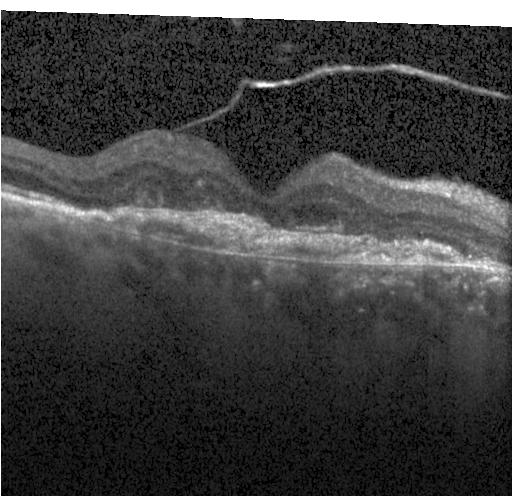

Retinal OCT B-scan
Diagnosis: a choroidal neovascular membrane.